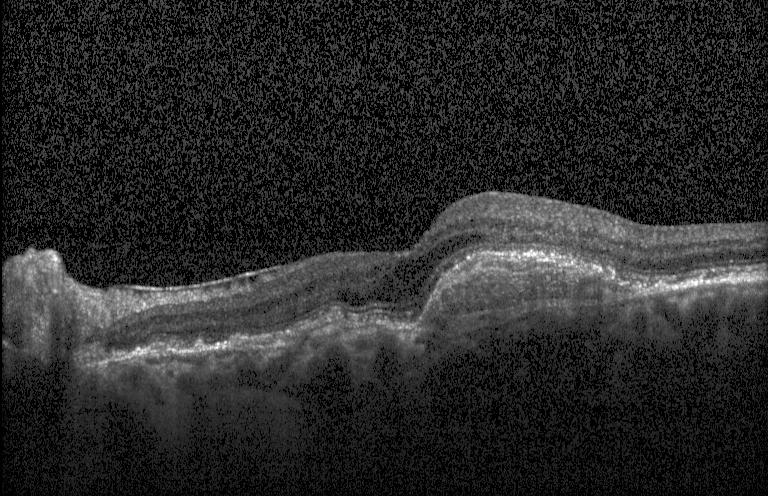
Diagnosis: a choroidal neovascular membrane.